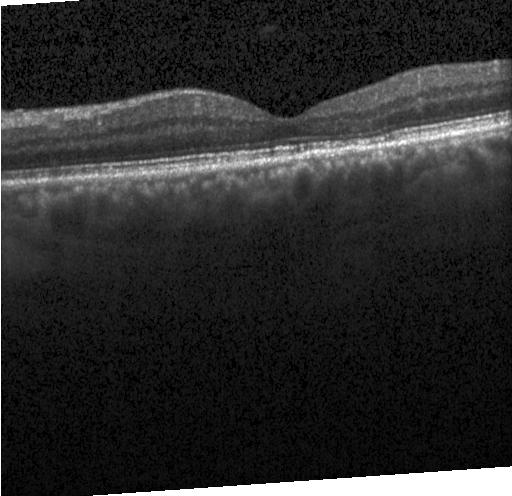 Optical coherence tomography B-scan — The scan shows no evidence of choroidal neovascularization, diabetic macular edema, or drusen.